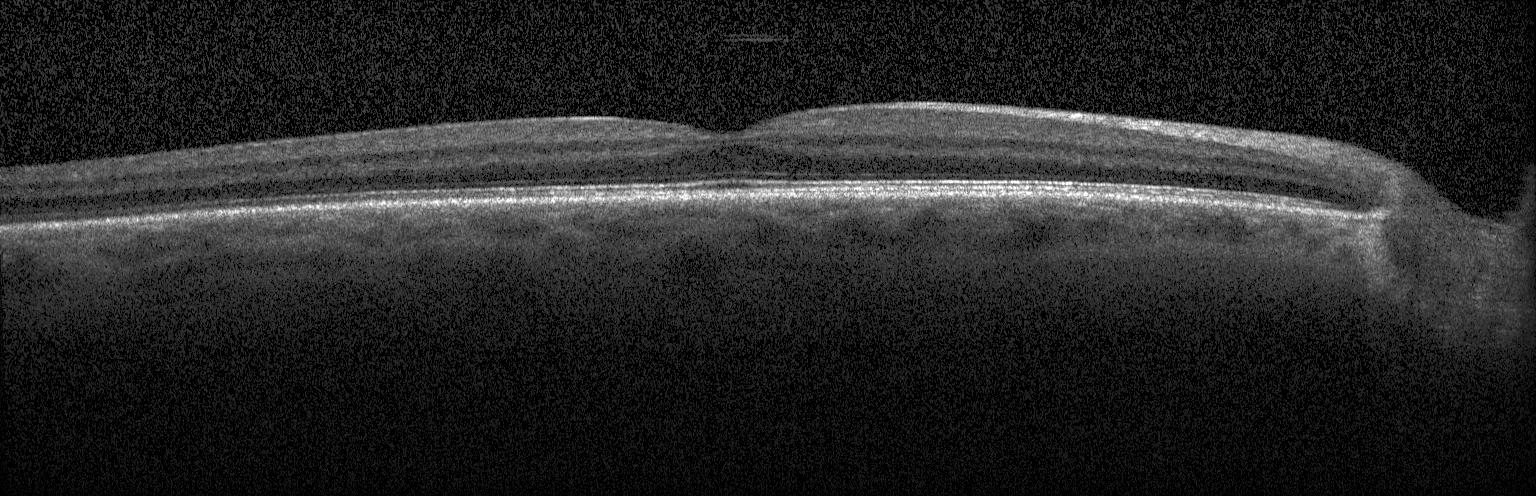
Horizontal scan through the fovea. Spectral-domain OCT. Instrument: Heidelberg Spectralis. Optical coherence tomography B-scan.
Diagnosis: no choroidal neovascularization, diabetic macular edema, or drusen.